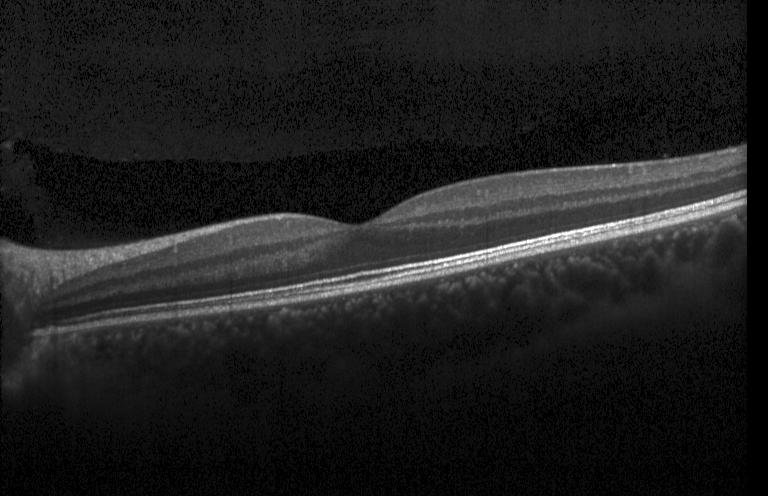
Instrument: Heidelberg Spectralis · centered on the fovea · retinal OCT B-scan
The scan shows neither CNV, DME, nor drusen.